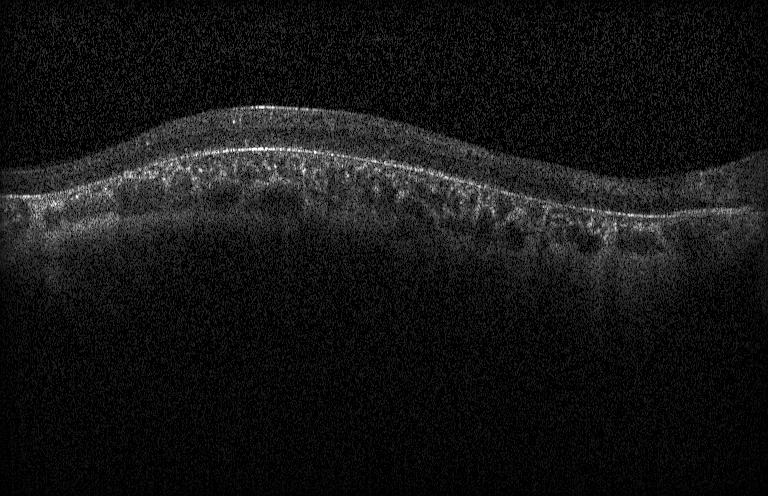
Instrument: Heidelberg Spectralis · retinal OCT cross-section.
No evidence of choroidal neovascularization, diabetic macular edema, or drusen.